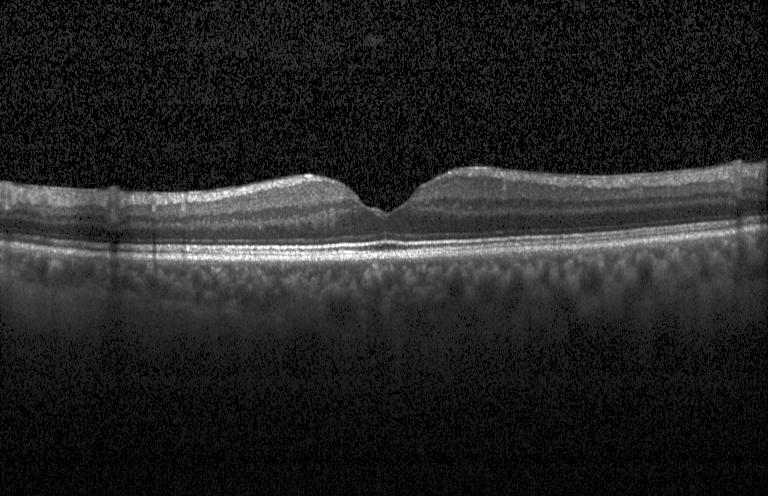

Diagnosis: neither choroidal neovascularization, diabetic macular edema, nor drusen.